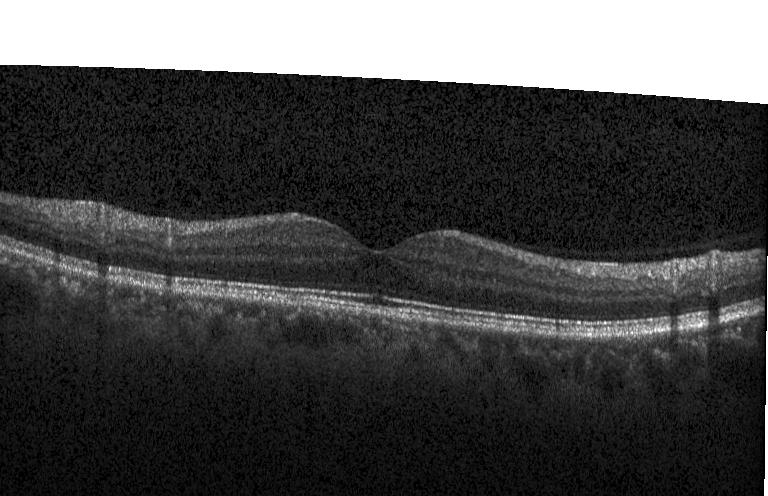
Optical coherence tomography B-scan.
Assessment: no CNV, DME, or drusen.